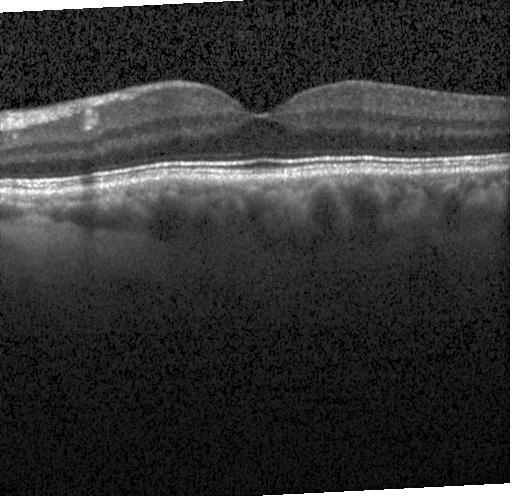

Retinal OCT cross-section showing no evidence of choroidal neovascularization, diabetic macular edema, or drusen.